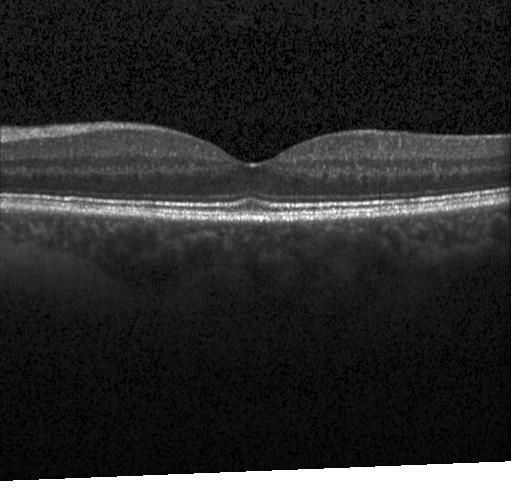

No choroidal neovascularization, no diabetic macular edema, and no drusen.